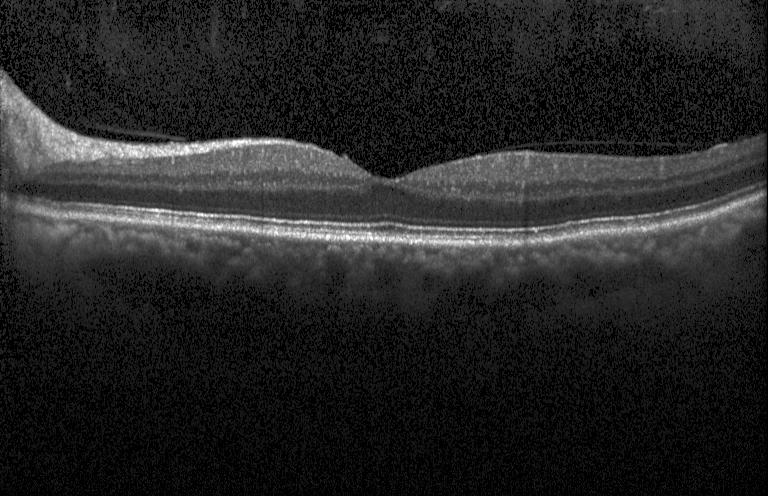 Optical coherence tomography B-scan · SD-OCT.
Impression: neither choroidal neovascularization, diabetic macular edema, nor drusen.